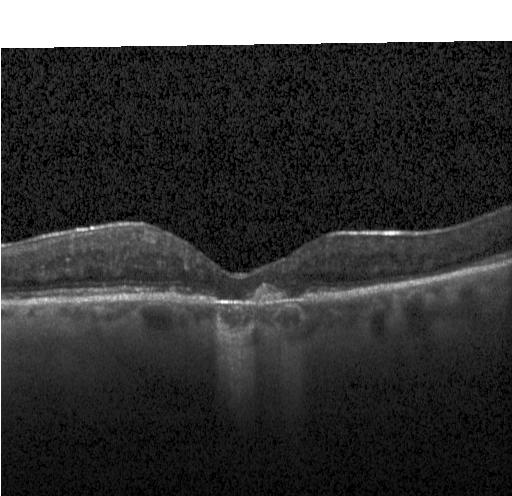
SD-OCT. Instrument: Heidelberg Spectralis. Retinal OCT B-scan. Through the macula
Assessment: a choroidal neovascular membrane.